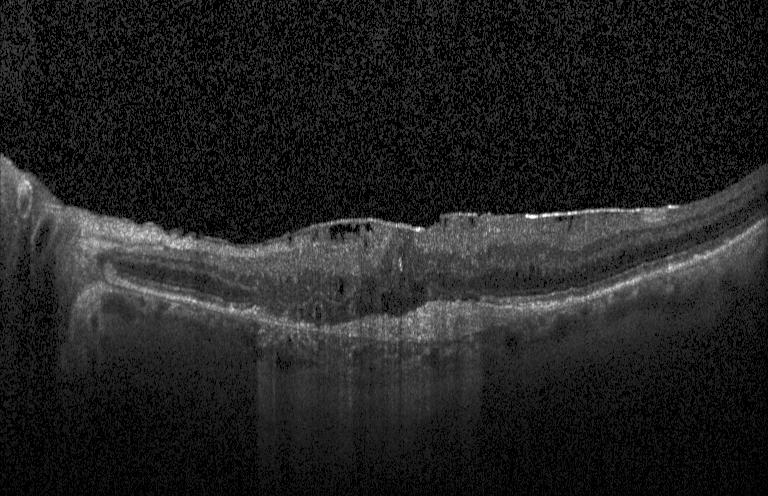 SD-OCT, retinal OCT cross-section. OCT finding: choroidal neovascularization (CNV).